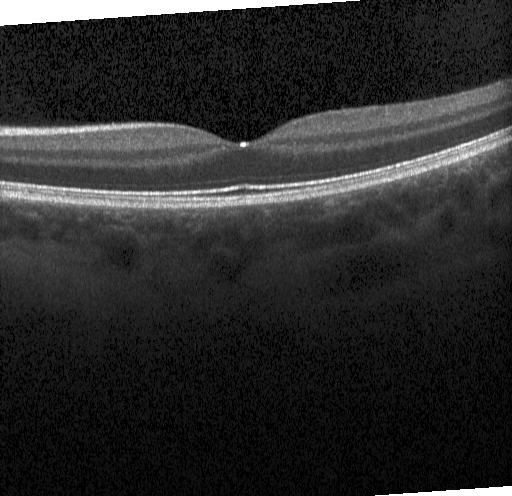 Finding: no choroidal neovascularization, diabetic macular edema, or drusen.